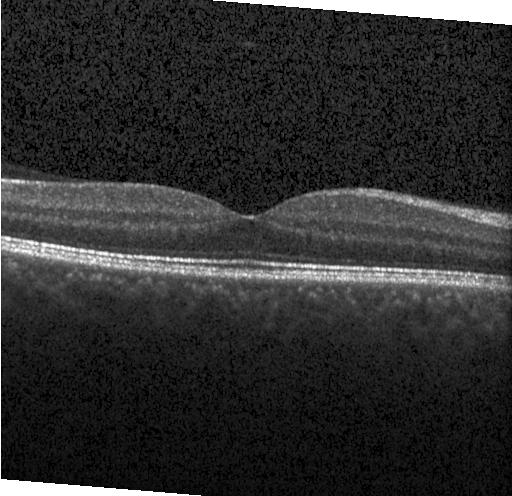

Instrument: Heidelberg Spectralis · OCT line scan · macular scan.
Diagnosis: no choroidal neovascularization, diabetic macular edema, or drusen.